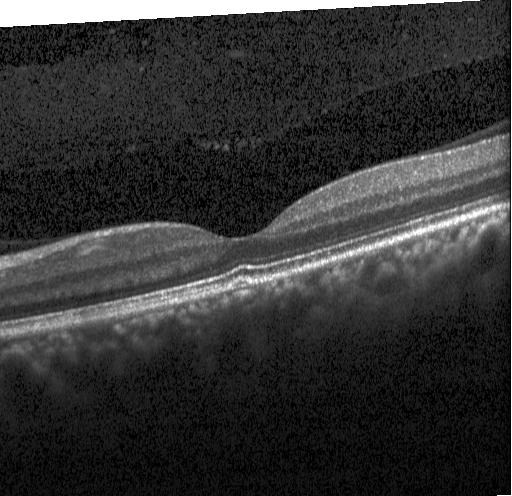

Retinal OCT cross-section; spectral-domain optical coherence tomography; instrument: Heidelberg Spectralis; horizontal scan through the fovea
Impression: drusen.